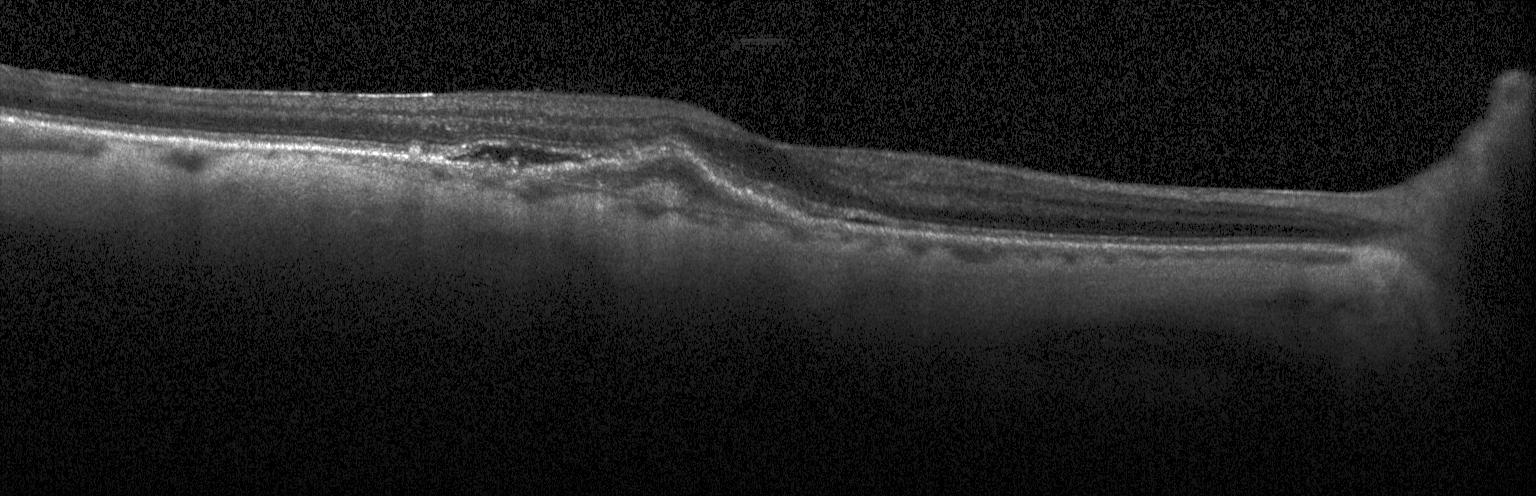 Dx: CNV.